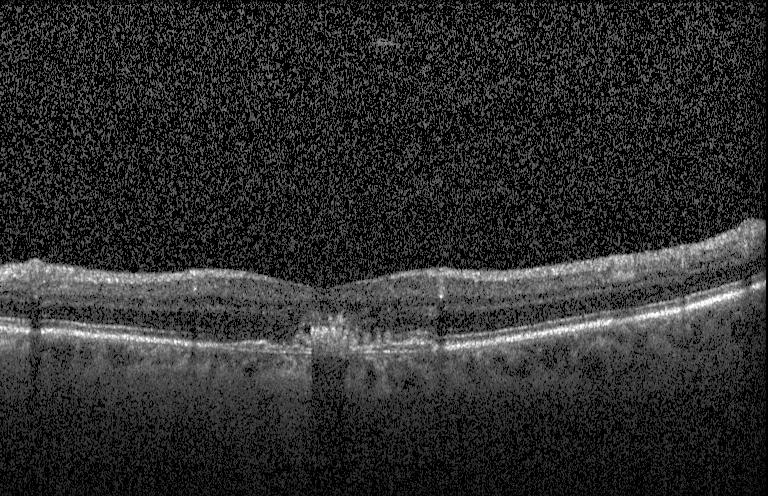
Dx: CNV.